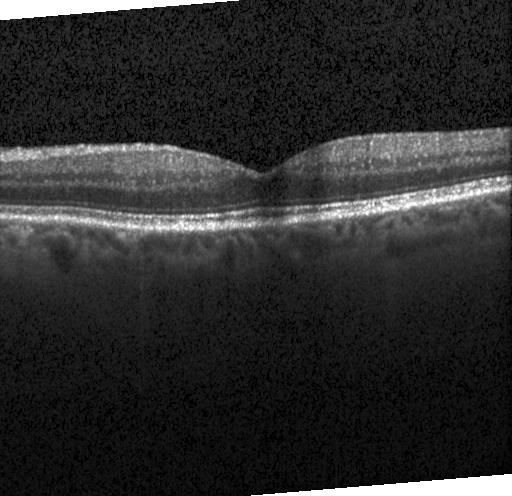 Finding: no choroidal neovascularization, no diabetic macular edema, and no drusen.